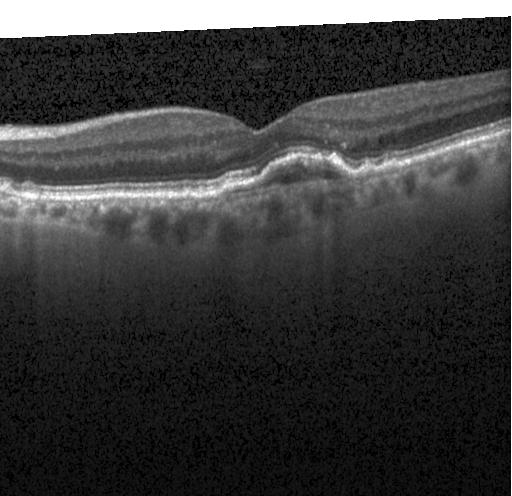

Spectral-domain optical coherence tomography, OCT B-scan, instrument: Heidelberg Spectralis — Impression: choroidal neovascularization (CNV).